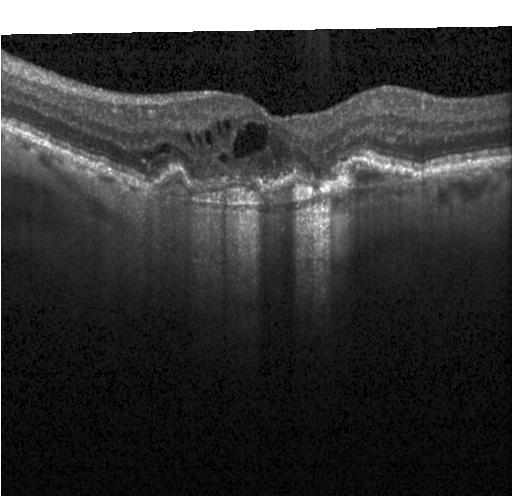

Finding: a choroidal neovascular membrane.